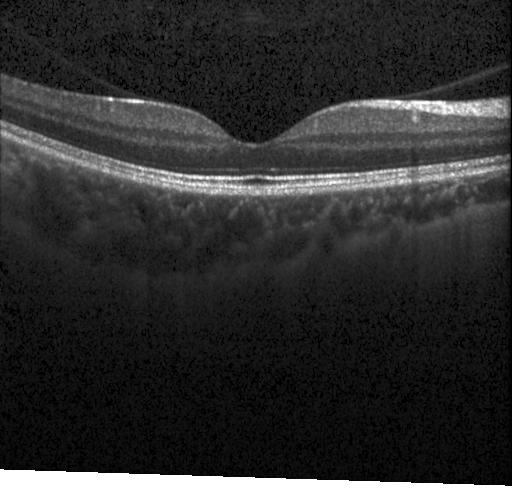 Fovea-centered. Spectral-domain OCT. Instrument: Heidelberg Spectralis. Optical coherence tomography scan. Finding: no CNV, DME, or drusen.